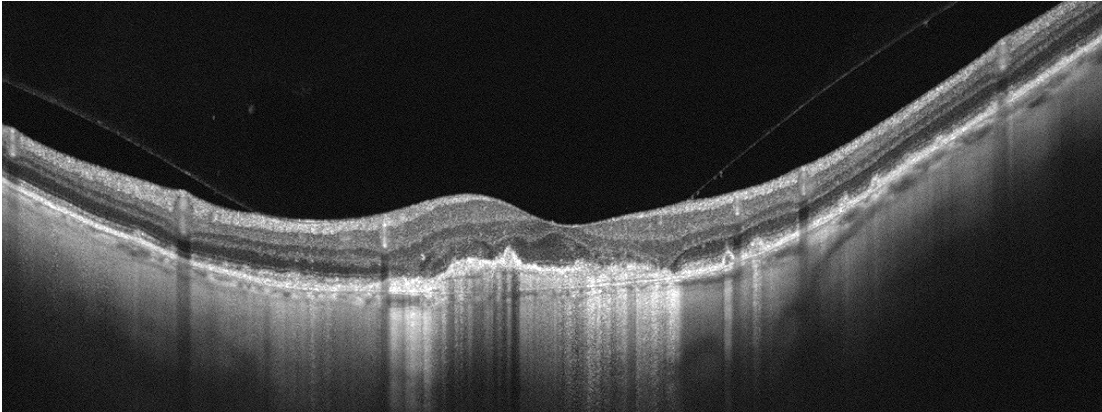

Through the macula, Optovue Avanti RTVue XR, retinal OCT cross-section.
This B-scan demonstrates AMD.